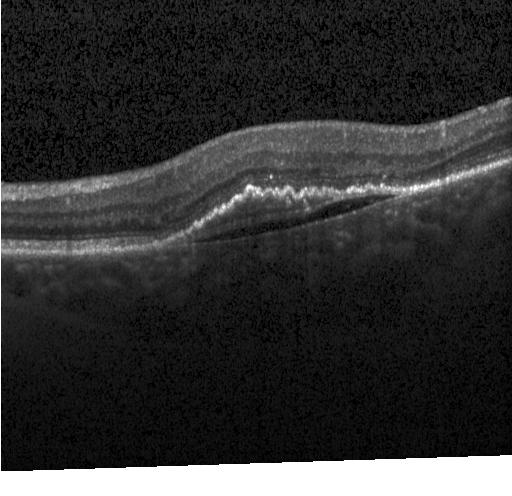 This B-scan demonstrates a choroidal neovascular membrane.